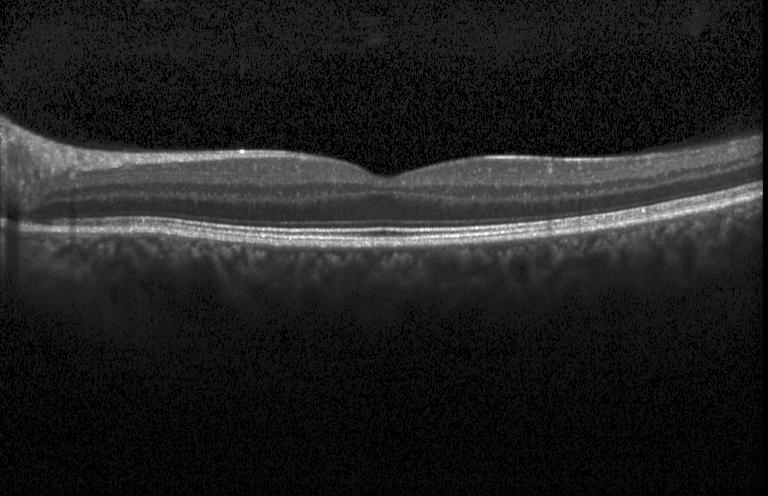 Centered on the fovea, optical coherence tomography scan.
Macular OCT: no CNV, DME, or drusen.